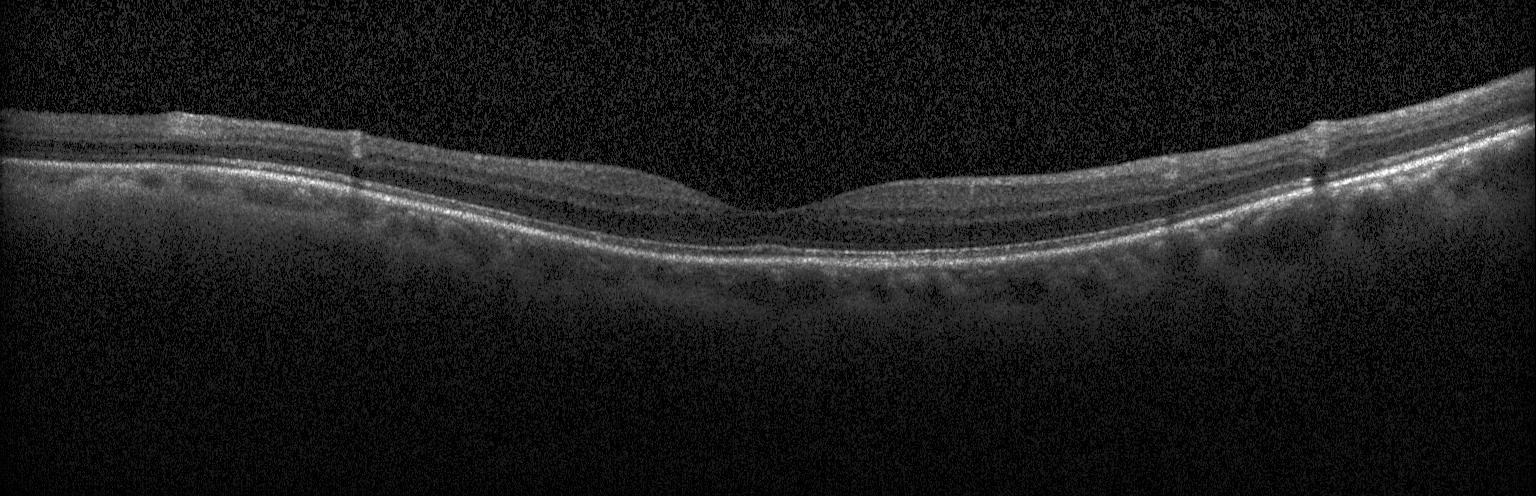 Heidelberg Spectralis OCT system, OCT line scan, horizontal scan through the fovea, SD-OCT. OCT finding: no choroidal neovascularization, no diabetic macular edema, and no drusen.